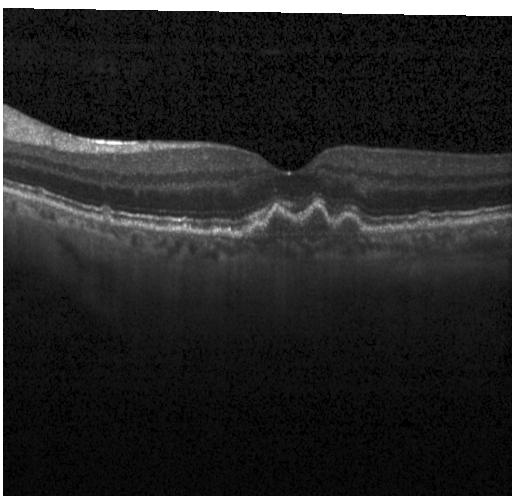
The scan shows multiple drusen.